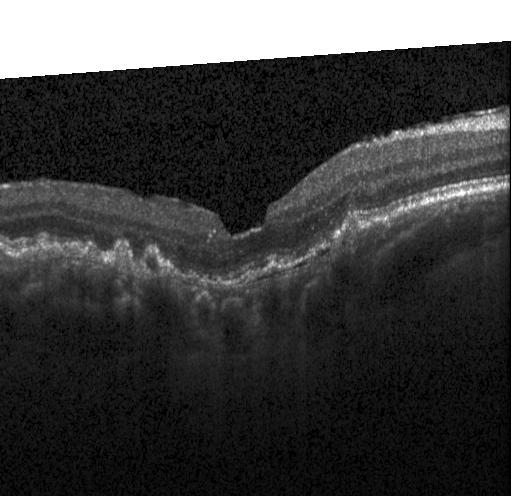 OCT B-scan, spectral-domain OCT
Finding: a choroidal neovascular membrane.